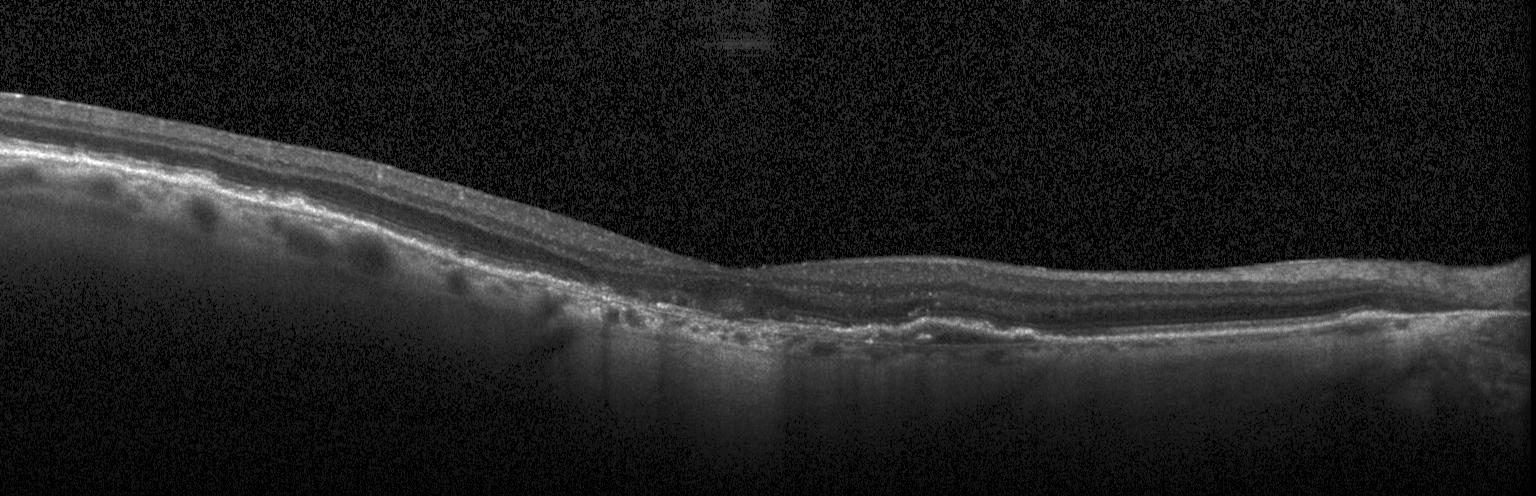

Heidelberg Spectralis OCT system; OCT line scan. Macular OCT: a choroidal neovascular membrane.